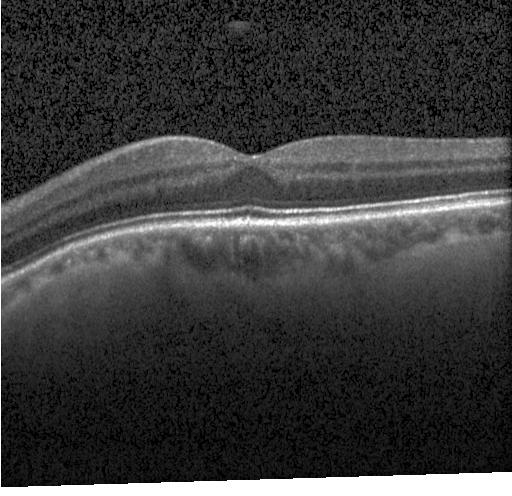

Finding: no choroidal neovascularization, diabetic macular edema, or drusen.